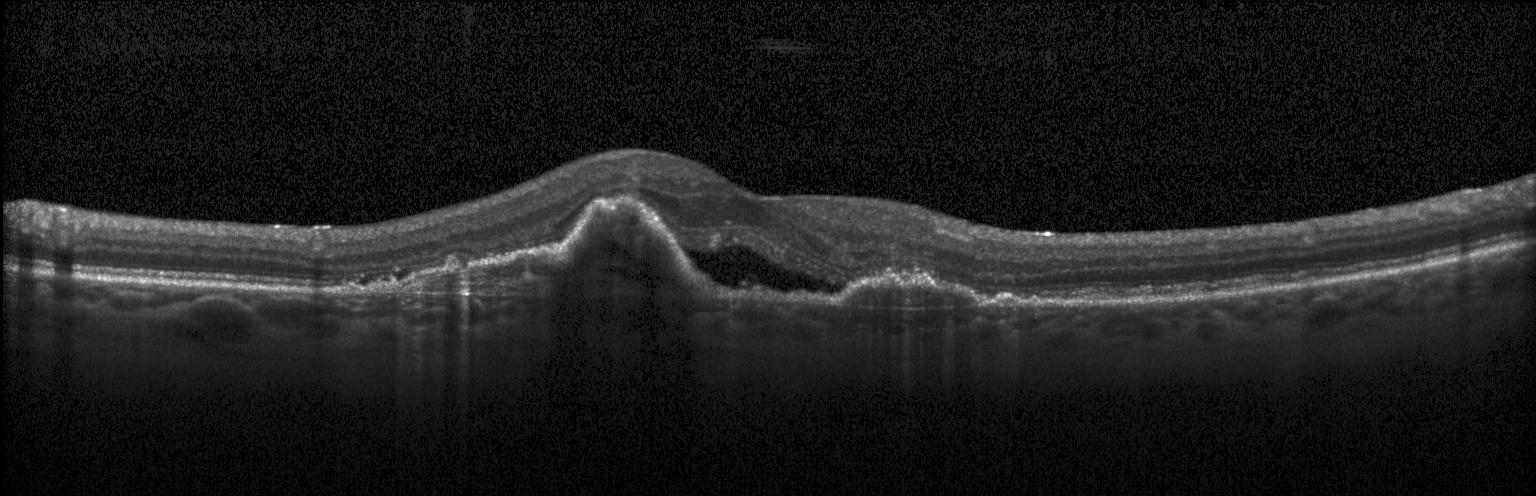

OCT B-scan; fovea-centered. Dx: choroidal neovascularization.